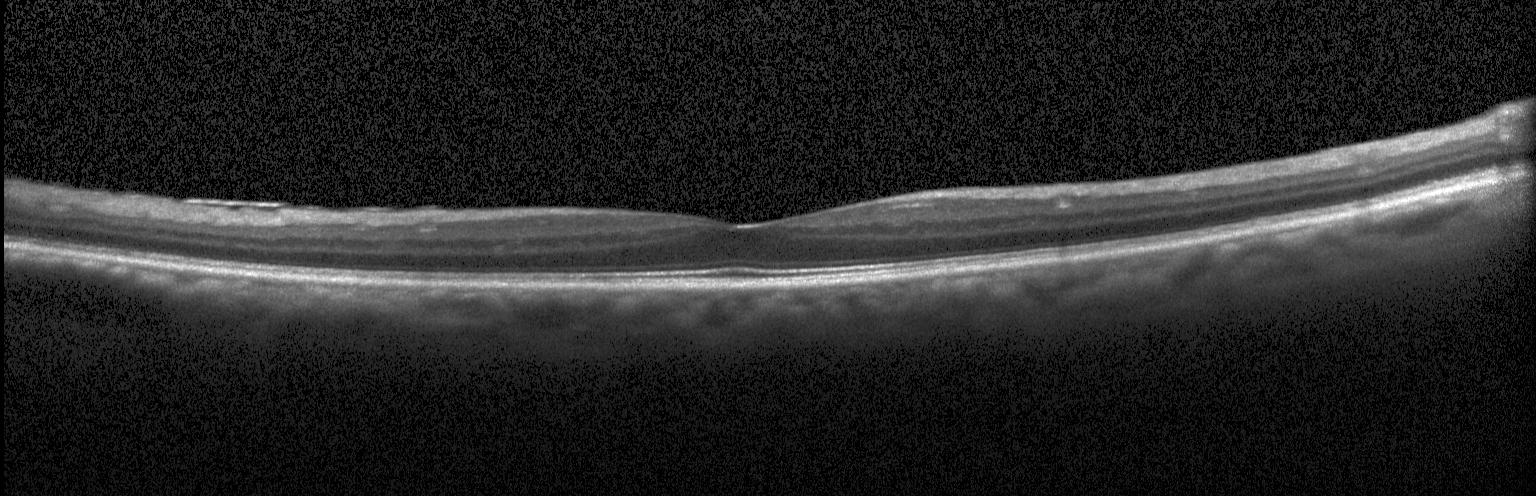 OCT B-scan · fovea-centered.
Finding: no choroidal neovascularization, diabetic macular edema, or drusen.